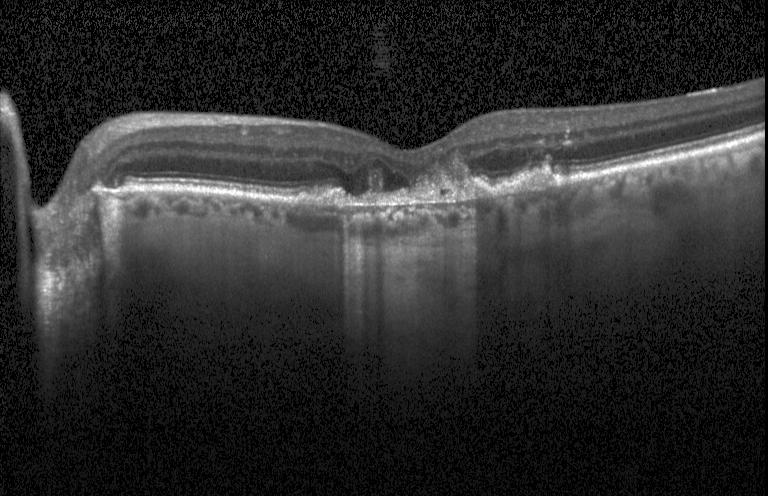 This B-scan demonstrates choroidal neovascularization (CNV).